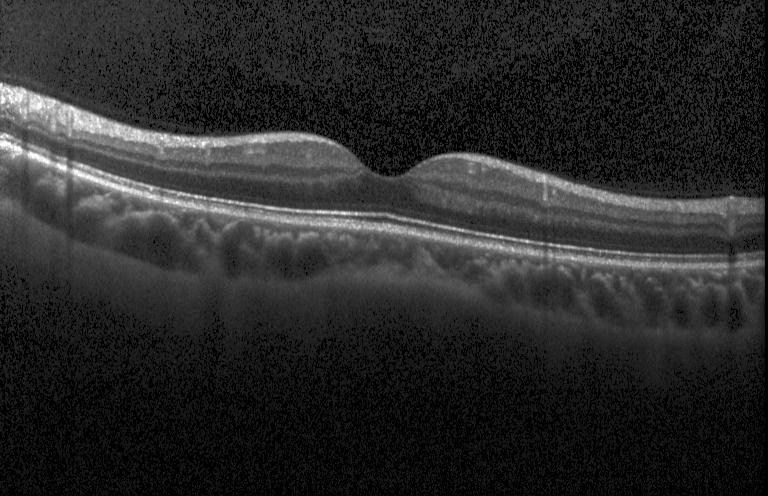

Retinal OCT cross-section, acquired on a Heidelberg Spectralis
Assessment: no choroidal neovascularization, diabetic macular edema, or drusen.